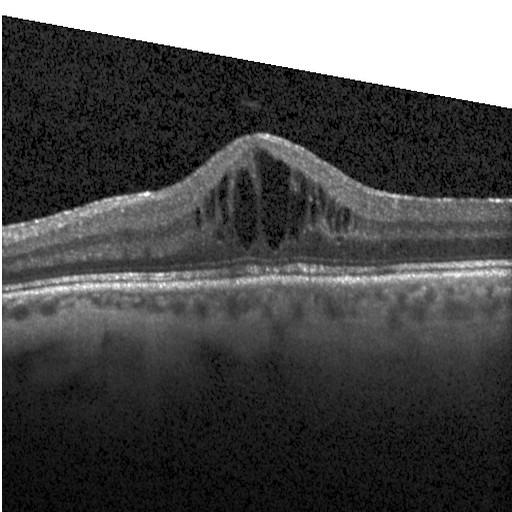

Retinal OCT cross-section, horizontal scan through the fovea, SD-OCT
Impression: diabetic macular edema.